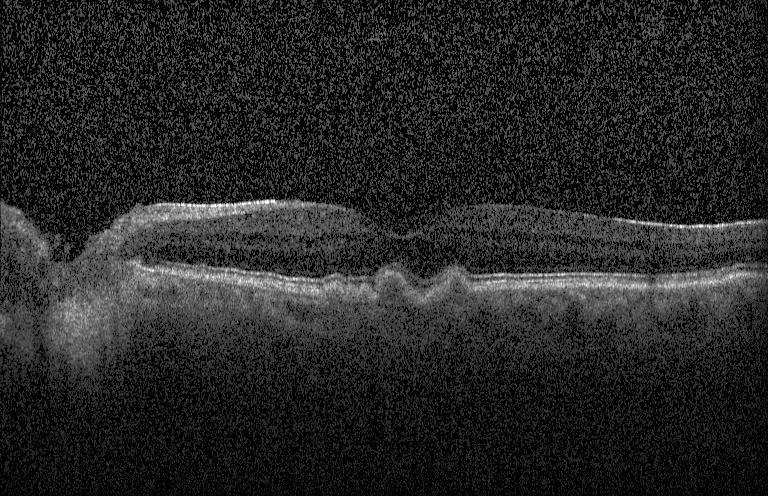

Through the macula. Acquired on a Heidelberg Spectralis. Optical coherence tomography B-scan. Diagnosis: sub-RPE drusenoid deposits.